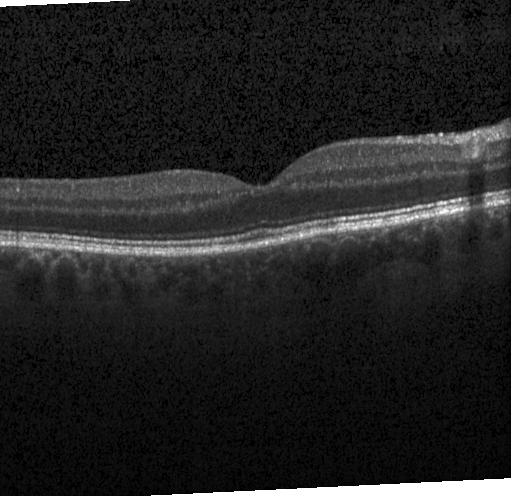

Spectral-domain OCT · retinal OCT B-scan
Finding: no evidence of choroidal neovascularization, diabetic macular edema, or drusen.